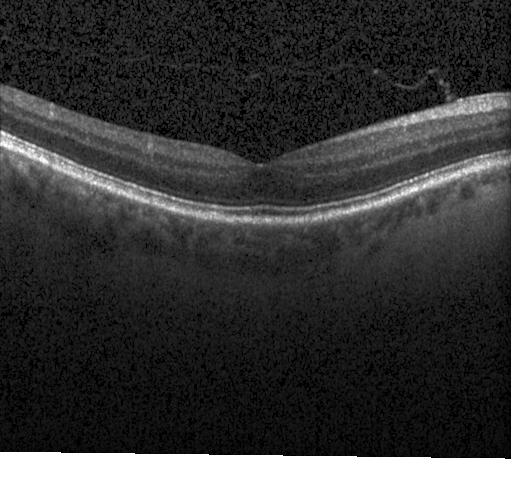
Diagnosis: no choroidal neovascularization, diabetic macular edema, or drusen.